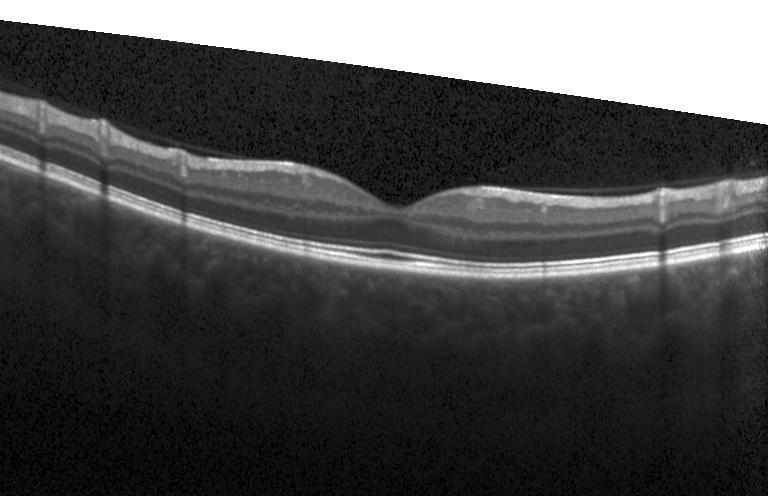 Optical coherence tomography scan, instrument: Heidelberg Spectralis. Macular OCT: no choroidal neovascularization, no diabetic macular edema, and no drusen.